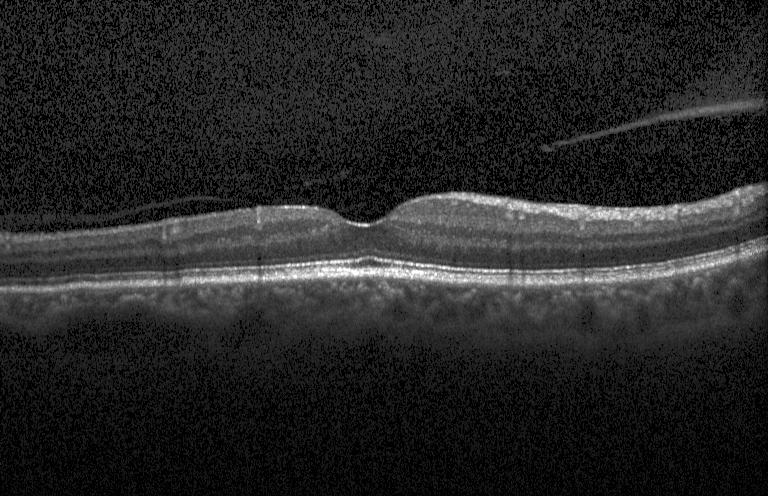 Finding: no CNV, no DME, and no drusen.